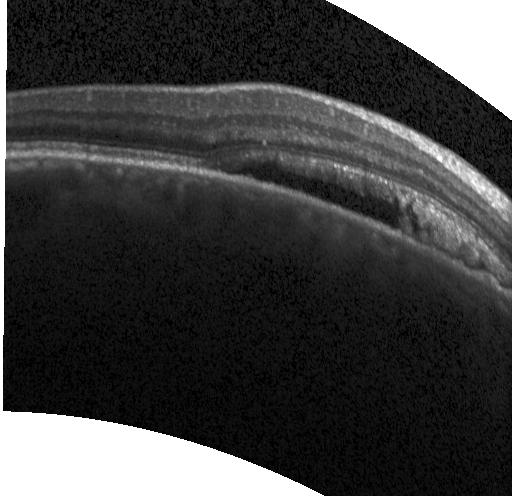
Diagnosis: choroidal neovascularization.